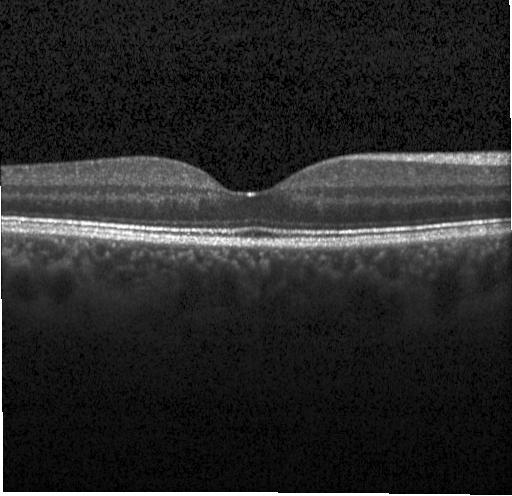

SD-OCT; optical coherence tomography scan; macular scan.
Finding: neither choroidal neovascularization, diabetic macular edema, nor drusen.